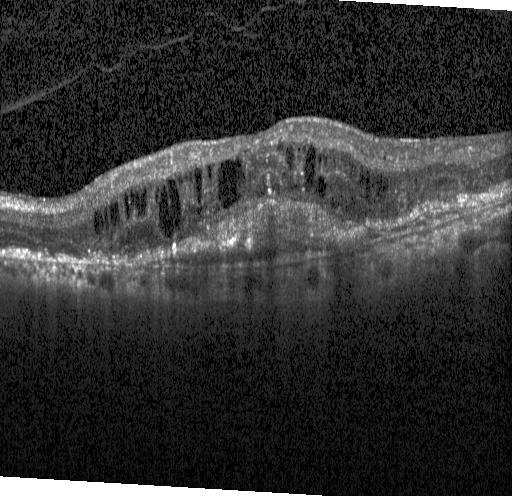
Retinal OCT B-scan; fovea-centered. Impression: choroidal neovascularization.